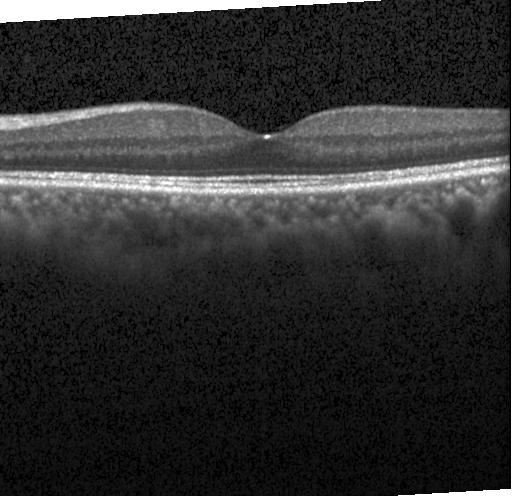
Centered on the fovea. Optical coherence tomography B-scan. Spectral-domain optical coherence tomography. Heidelberg Spectralis
OCT finding: neither choroidal neovascularization, diabetic macular edema, nor drusen.